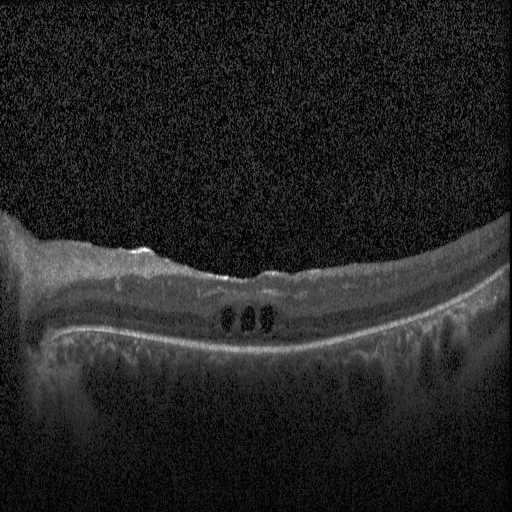
Retinal OCT cross-section showing diabetic macular edema (DME).